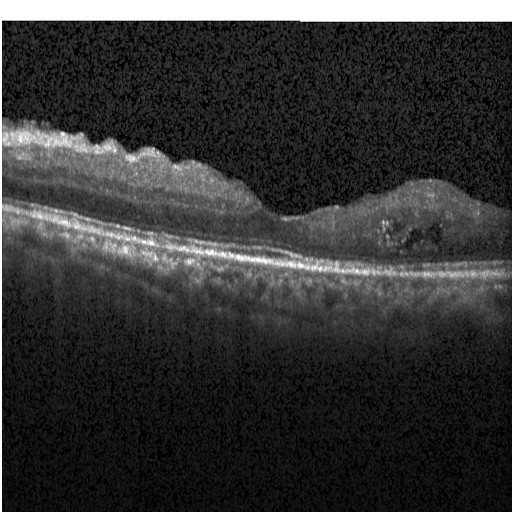
This B-scan demonstrates DME.